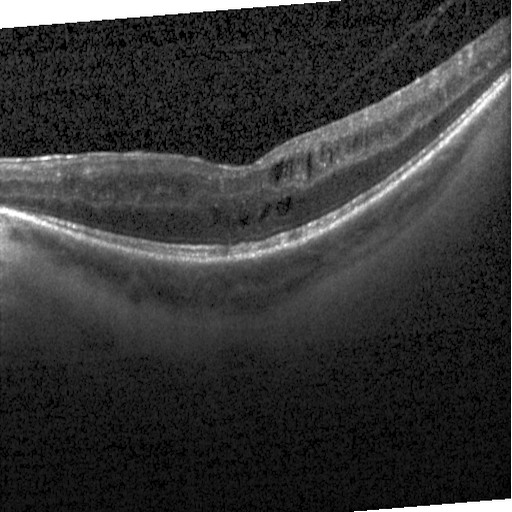 OCT B-scan, horizontal scan through the fovea, Heidelberg Spectralis OCT system.
Diagnosis: DME.